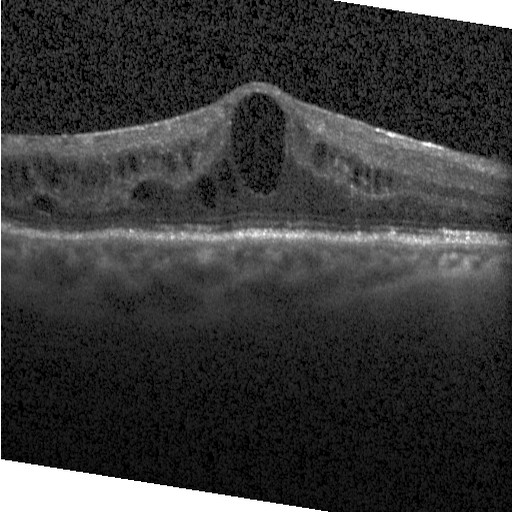

The scan shows diabetic macular edema.